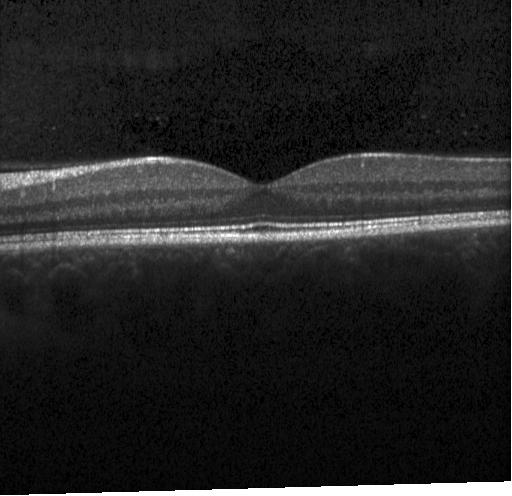
Assessment: no choroidal neovascularization, no diabetic macular edema, and no drusen.